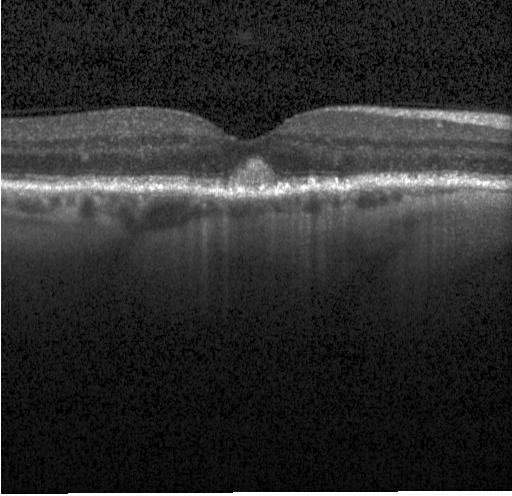
Dx: drusen.